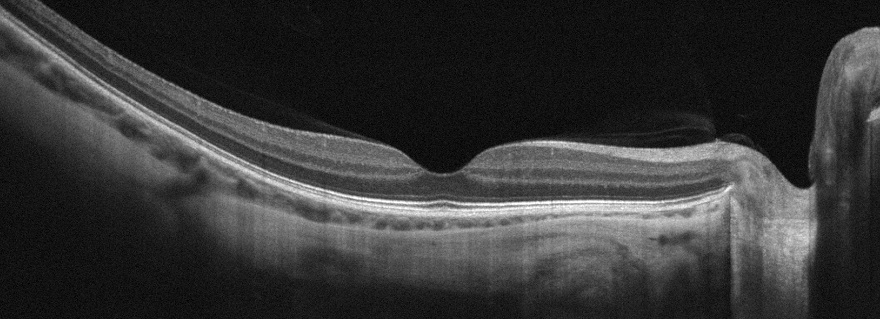

Optical coherence tomography scan; through the macula
Finding: no AMD, DME, ERM, RAO, RVO, or VID.